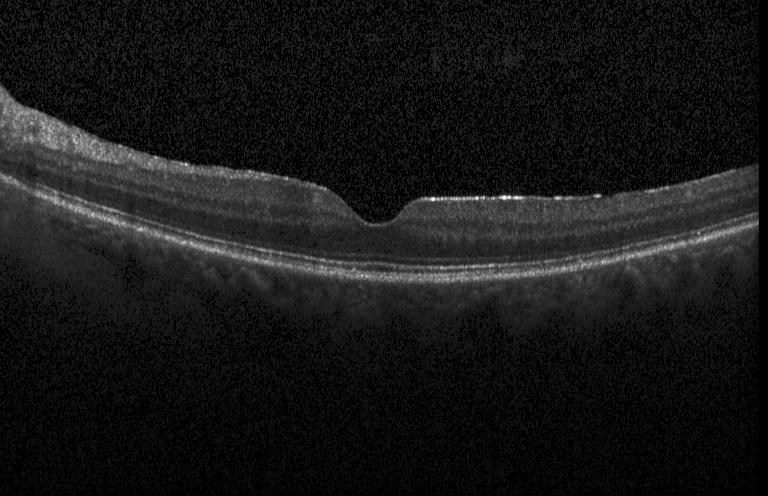

Finding: no choroidal neovascularization, no diabetic macular edema, and no drusen.